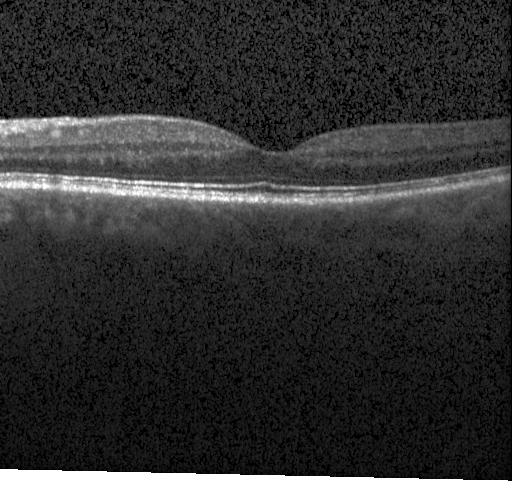
Heidelberg Spectralis. Spectral-domain OCT. Optical coherence tomography B-scan. The scan shows neither choroidal neovascularization, diabetic macular edema, nor drusen.